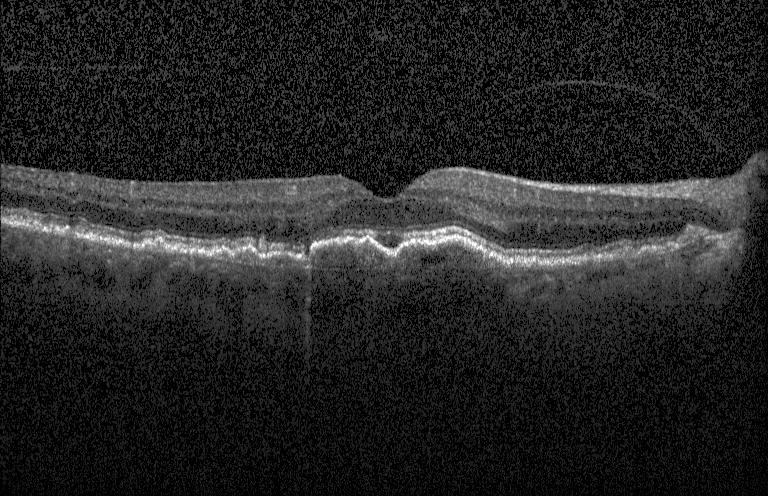 Impression: choroidal neovascularization.